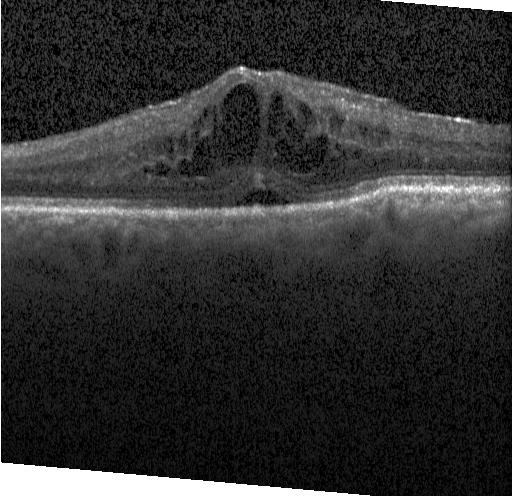
Acquired on a Heidelberg Spectralis, retinal OCT B-scan, fovea-centered. OCT finding: diabetic macular edema (DME).